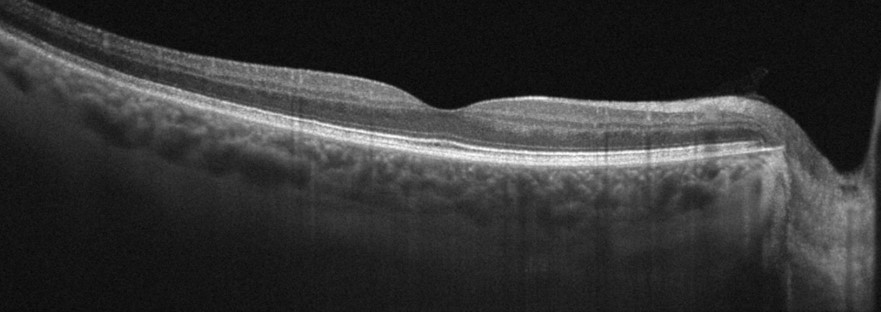
Retinal OCT cross-section; Optovue Avanti RTVue XR.
This B-scan demonstrates no AMD, DME, ERM, RAO, RVO, or VID.